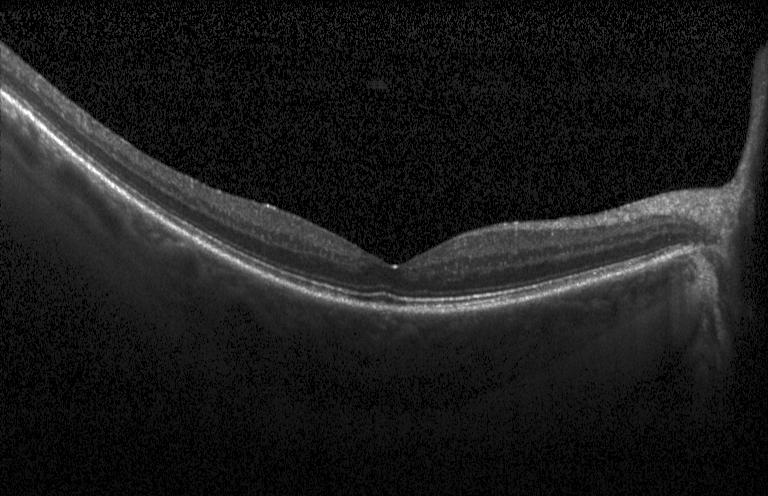

Finding: neither choroidal neovascularization, diabetic macular edema, nor drusen.